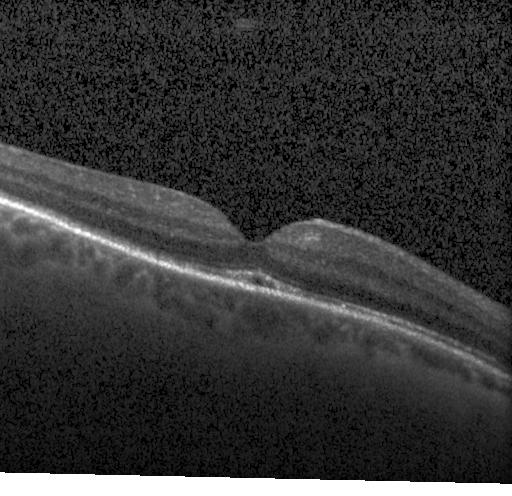

Centered on the fovea, instrument: Heidelberg Spectralis, optical coherence tomography scan. This B-scan demonstrates no choroidal neovascularization, diabetic macular edema, or drusen.